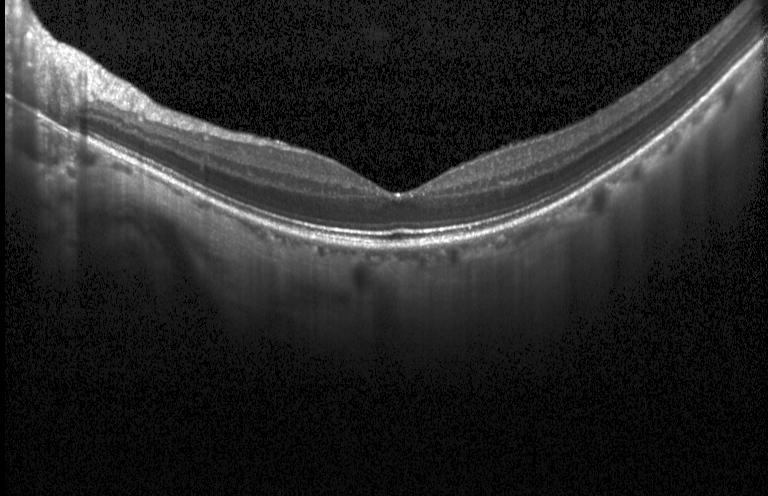
Spectral-domain OCT; retinal OCT B-scan; centered on the fovea; instrument: Heidelberg Spectralis
Assessment: neither choroidal neovascularization, diabetic macular edema, nor drusen.